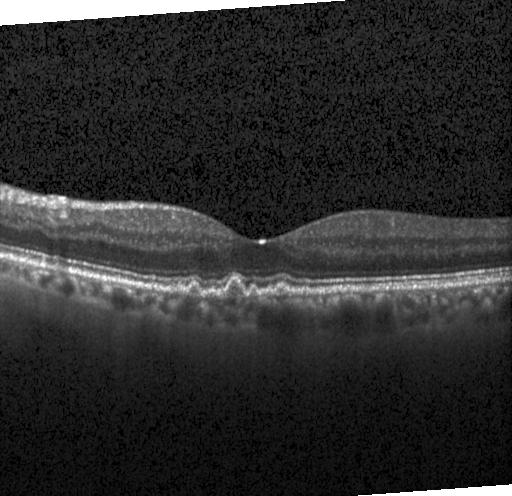
Spectral-domain OCT. OCT B-scan
Impression: sub-RPE drusenoid deposits.